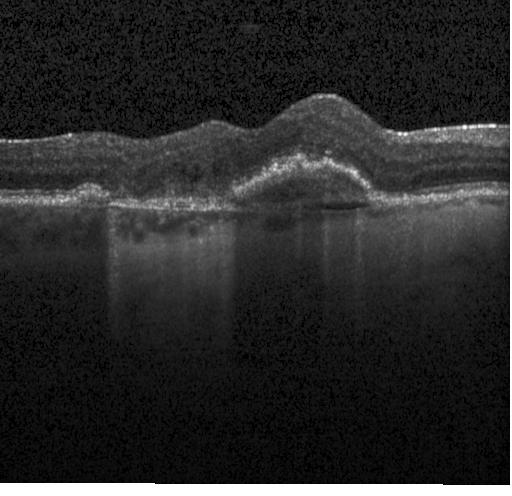
OCT line scan; SD-OCT. Finding: CNV.